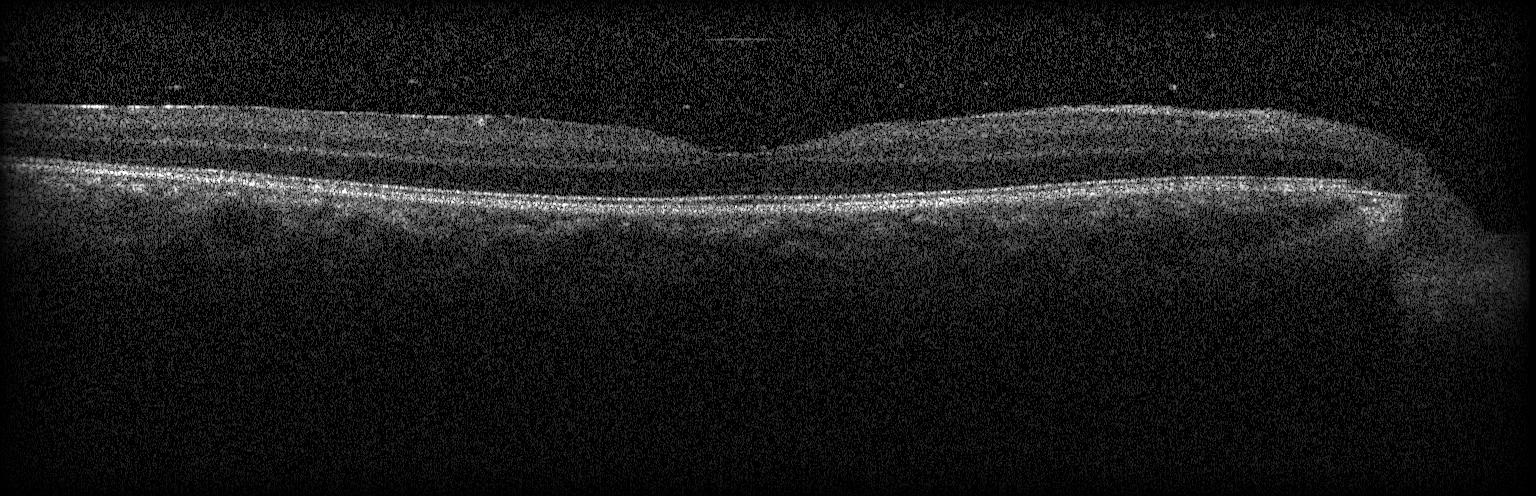
Optical coherence tomography B-scan · macular scan — Assessment: no choroidal neovascularization, no diabetic macular edema, and no drusen.